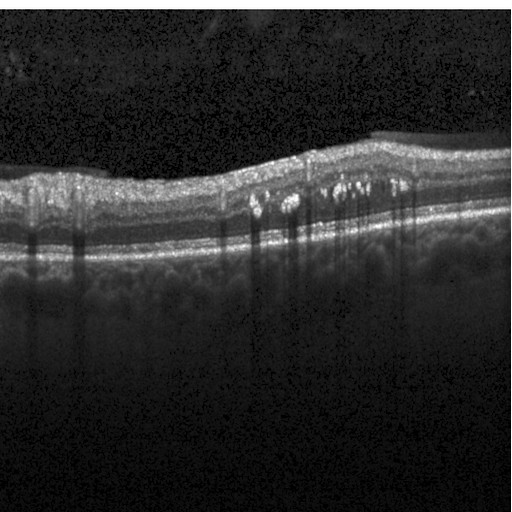 Horizontal scan through the fovea, spectral-domain optical coherence tomography, retinal OCT cross-section, acquired on a Heidelberg Spectralis
This B-scan demonstrates diabetic macular edema (DME).